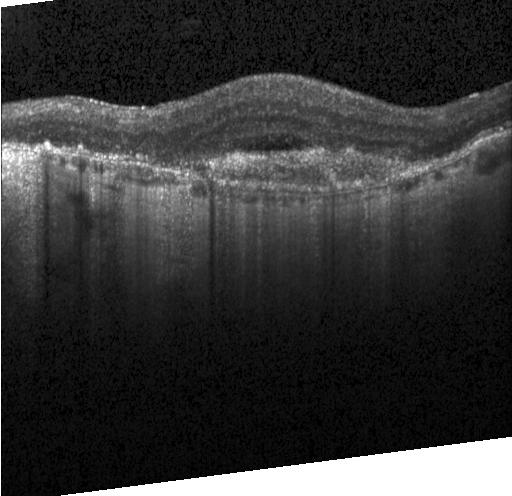
Optical coherence tomography B-scan · SD-OCT · centered on the fovea. Dx: a choroidal neovascular membrane.